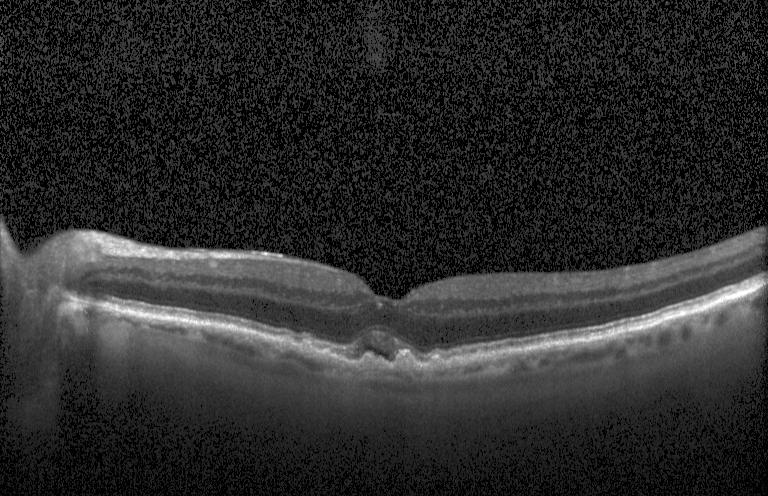

Dx: CNV.